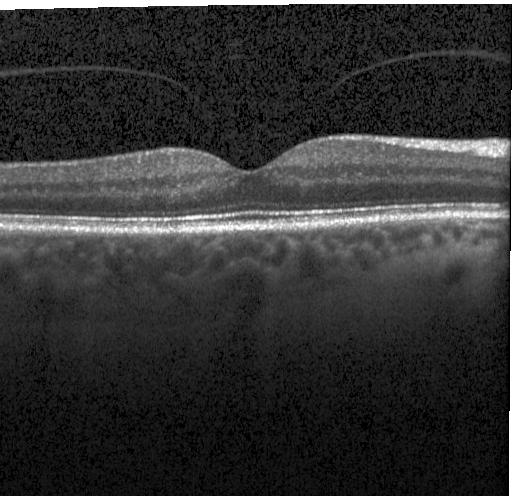

Dx: neither choroidal neovascularization, diabetic macular edema, nor drusen.